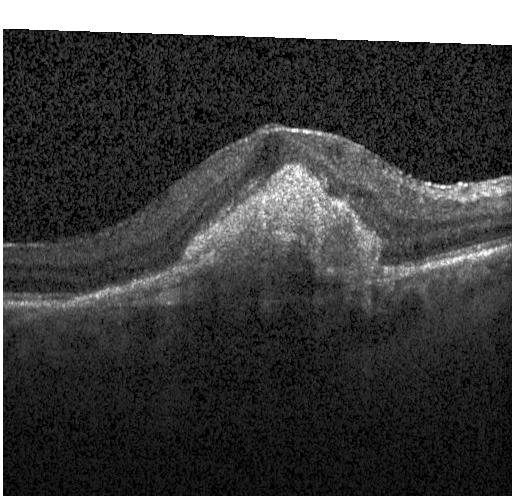 Spectral-domain OCT. Heidelberg Spectralis OCT system. Optical coherence tomography B-scan
Finding: a choroidal neovascular membrane.